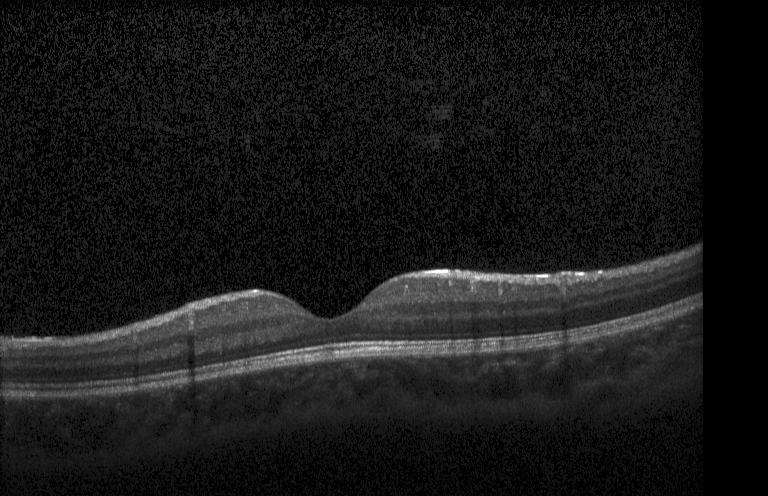 This B-scan demonstrates neither CNV, DME, nor drusen.